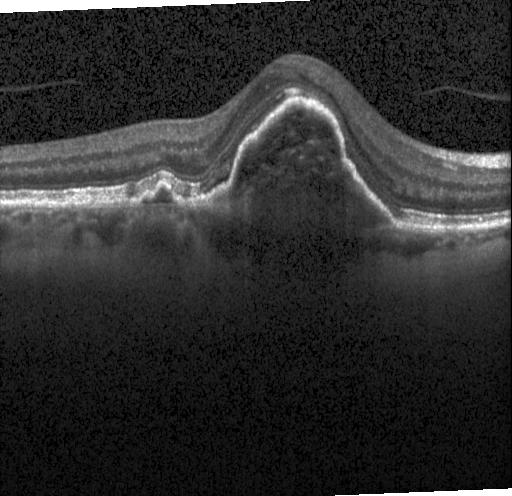 Retinal OCT cross-section. Dx: a choroidal neovascular membrane.